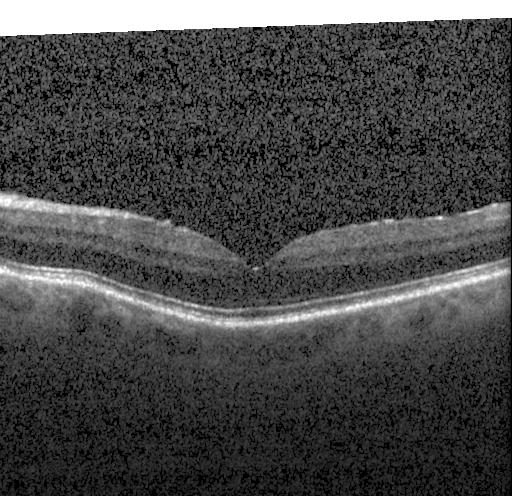

Optical coherence tomography B-scan.
This B-scan demonstrates no choroidal neovascularization, diabetic macular edema, or drusen.